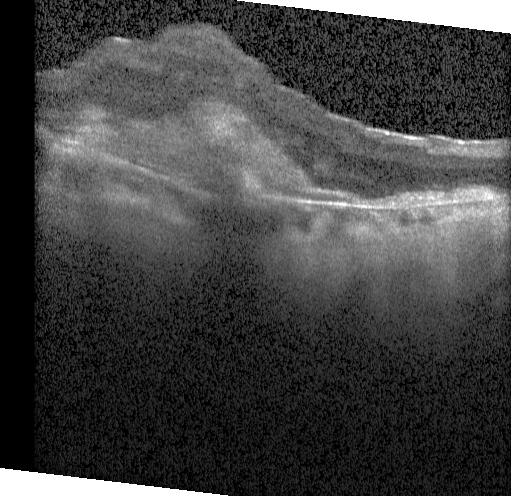
Finding: choroidal neovascularization (CNV).